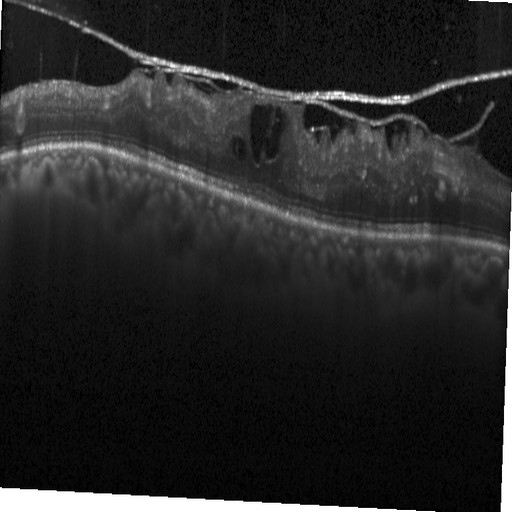 OCT line scan, instrument: Heidelberg Spectralis.
OCT finding: diabetic macular edema (DME).